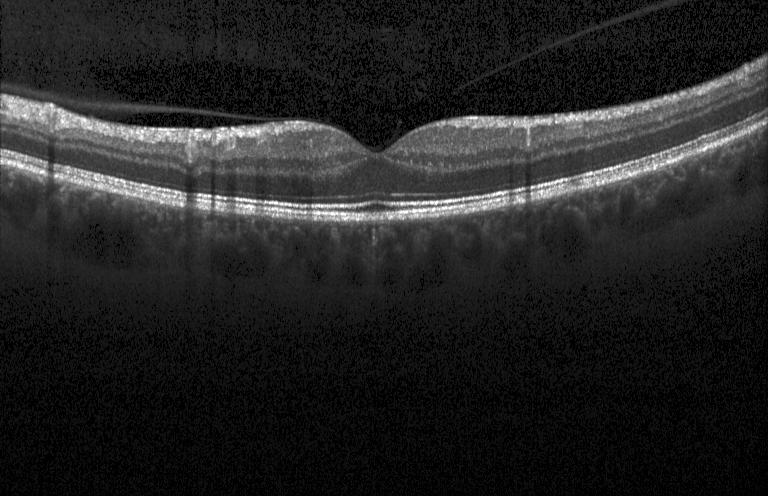

Spectral-domain OCT. OCT line scan. Heidelberg Spectralis OCT system.
Neither CNV, DME, nor drusen.